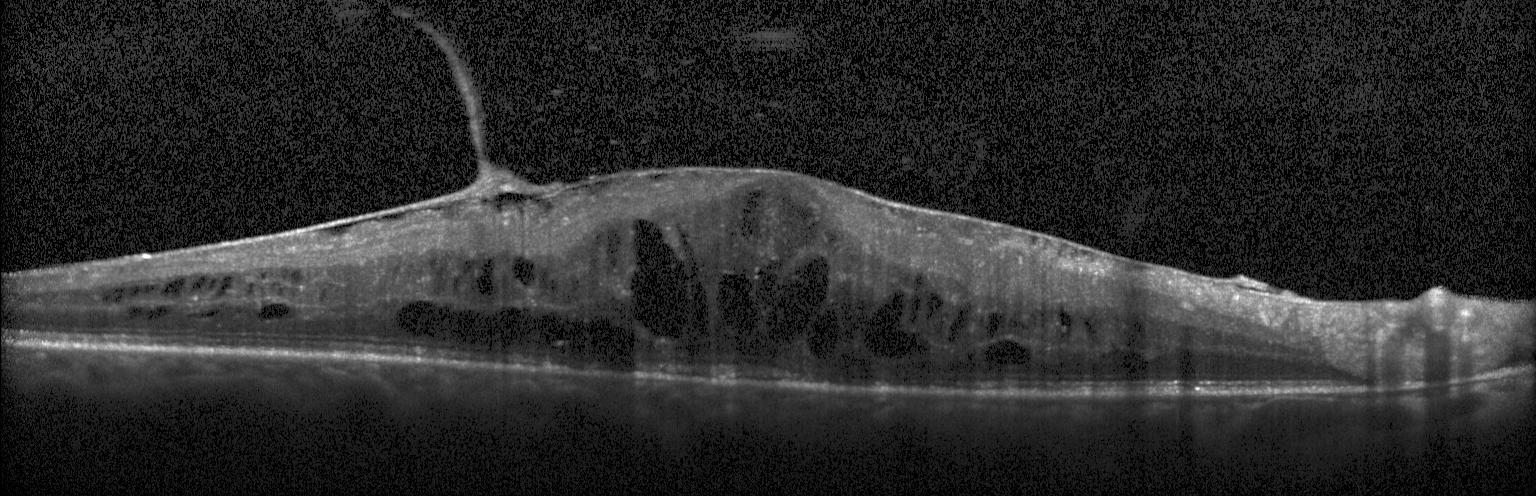 Impression: DME.